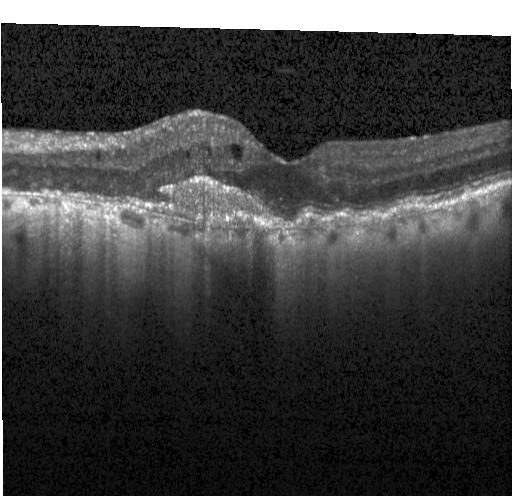

Retinal OCT cross-section · macular scan · Heidelberg Spectralis OCT system · spectral-domain OCT.
Finding: choroidal neovascularization.